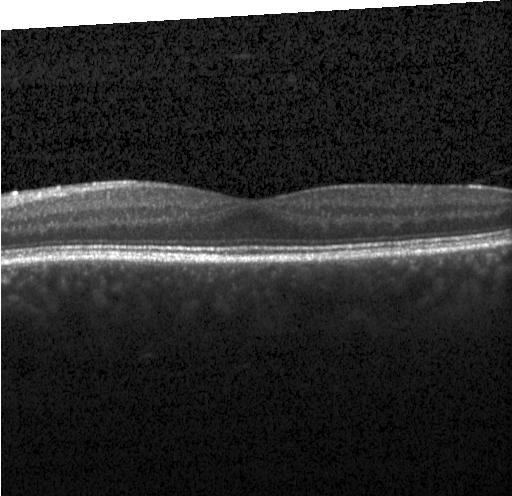
Optical coherence tomography scan · macular scan
No evidence of choroidal neovascularization, diabetic macular edema, or drusen.